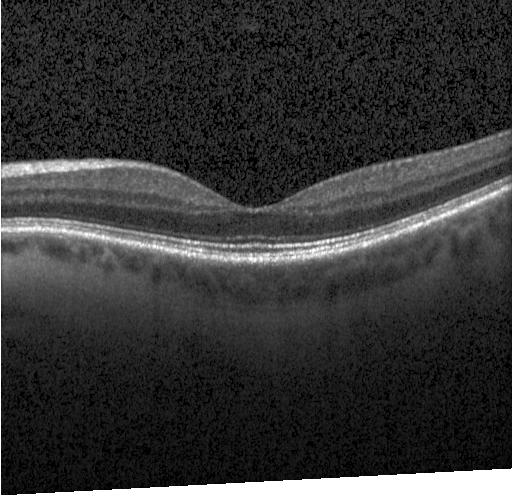
Retinal OCT cross-section.
Diagnosis: no choroidal neovascularization, diabetic macular edema, or drusen.